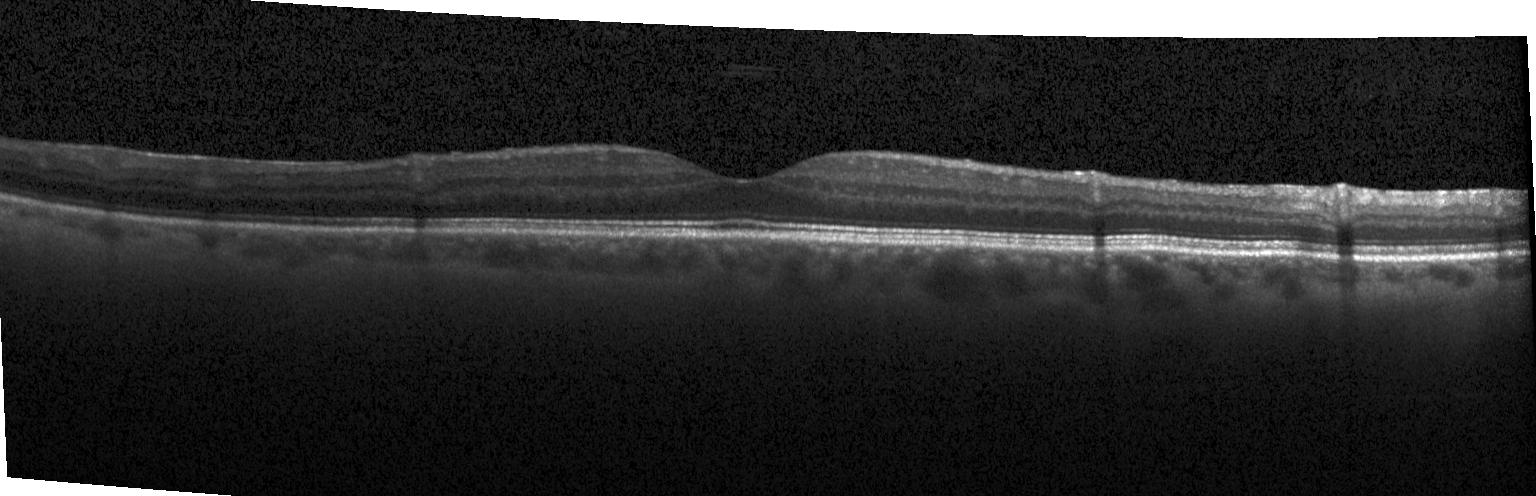 Impression: no CNV, no DME, and no drusen.